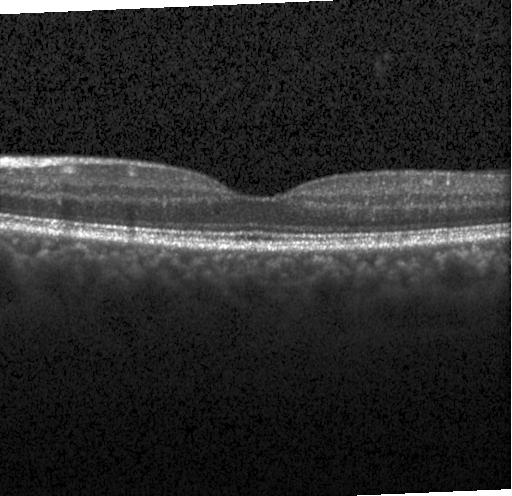 OCT B-scan — Impression: no choroidal neovascularization, diabetic macular edema, or drusen.